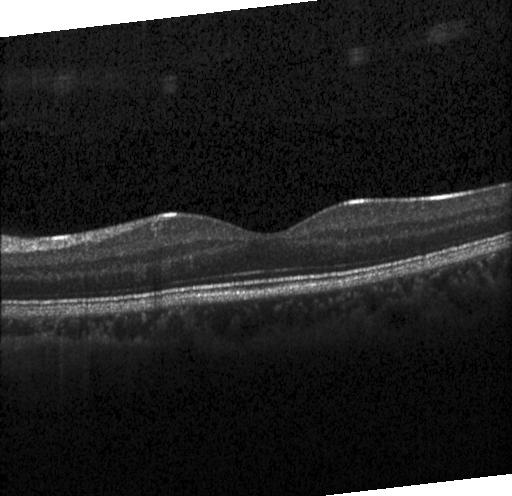
Optical coherence tomography B-scan; spectral-domain OCT — Dx: no evidence of CNV, DME, or drusen.